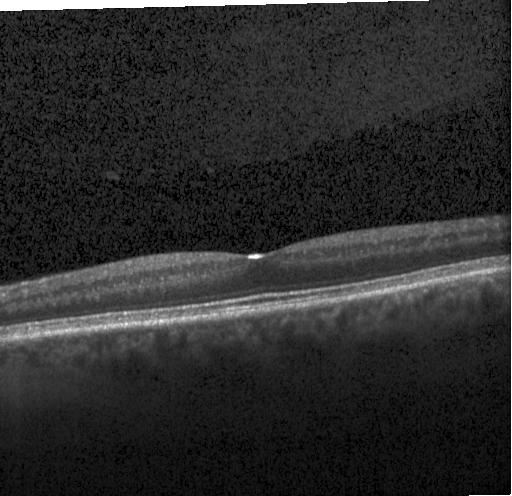
OCT finding: no evidence of choroidal neovascularization, diabetic macular edema, or drusen.